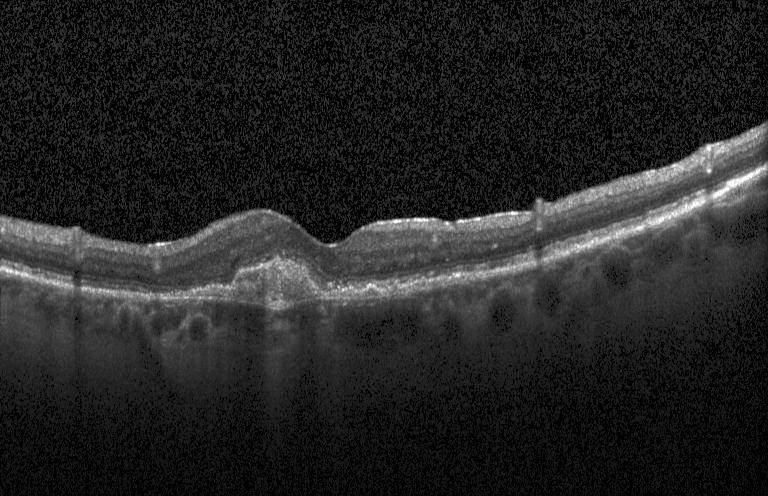 Retinal OCT cross-section showing CNV.